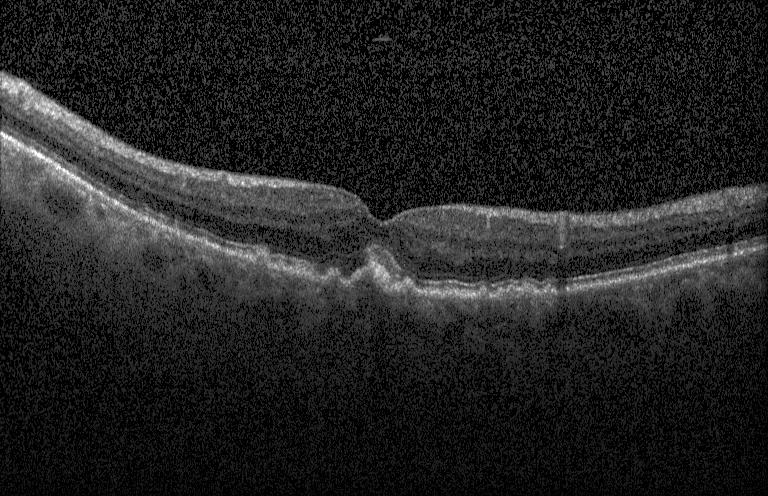

Optical coherence tomography B-scan. Assessment: sub-RPE drusenoid deposits.